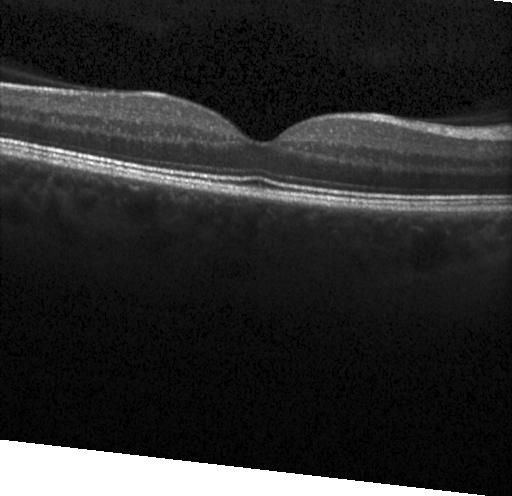
Finding: no CNV, no DME, and no drusen.